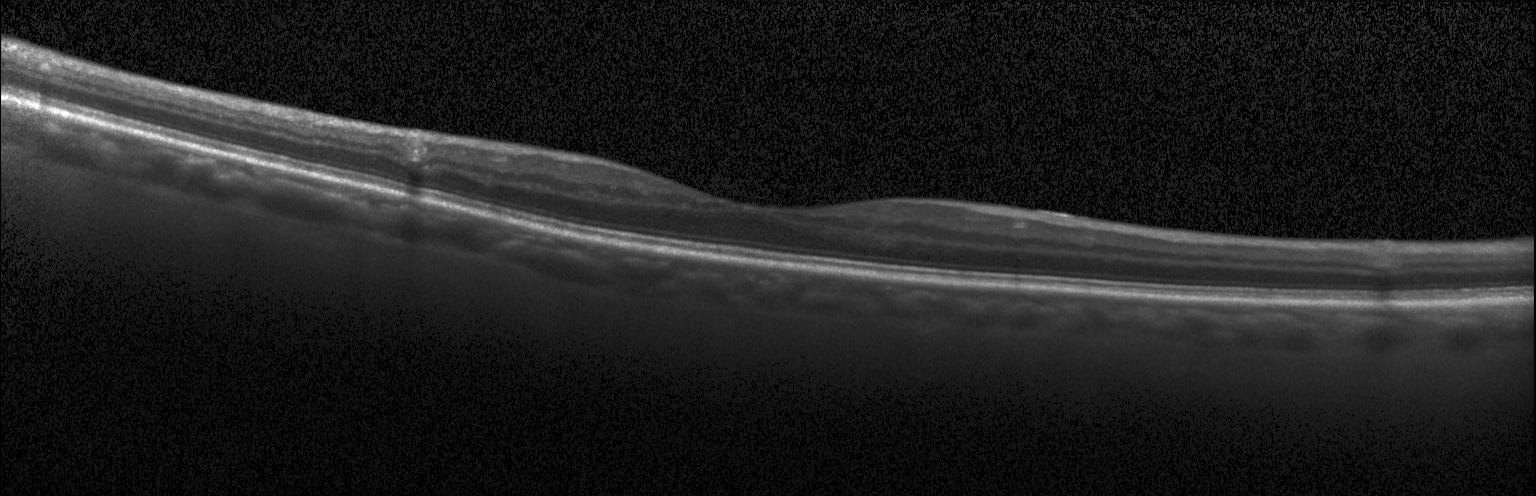
Optical coherence tomography B-scan — Assessment: neither choroidal neovascularization, diabetic macular edema, nor drusen.